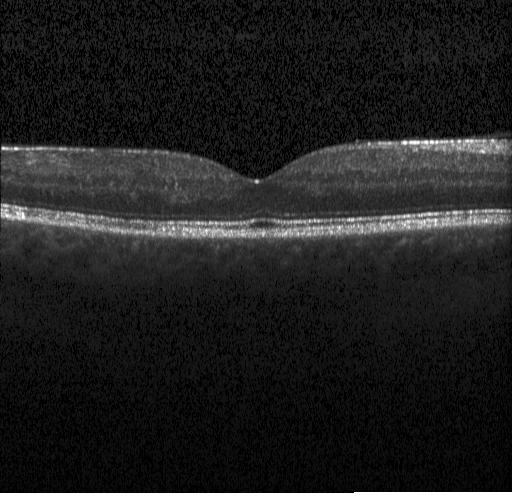
Macular scan · optical coherence tomography scan · spectral-domain optical coherence tomography. Assessment: no CNV, no DME, and no drusen.